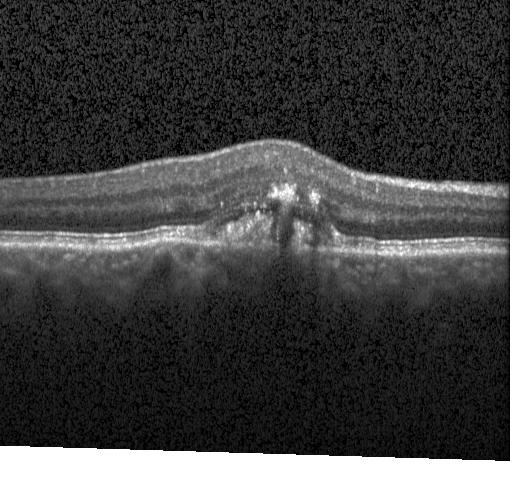
Finding: a choroidal neovascular membrane.